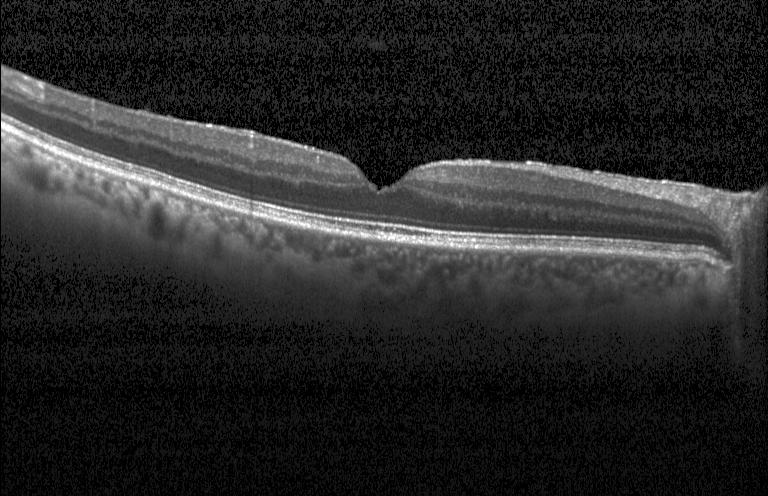

Retinal OCT B-scan.
Diagnosis: no choroidal neovascularization, no diabetic macular edema, and no drusen.